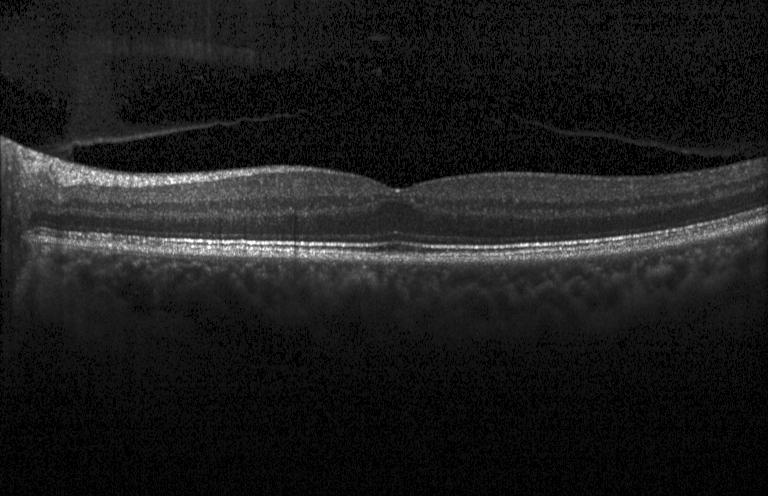 Optical coherence tomography scan. Impression: no evidence of choroidal neovascularization, diabetic macular edema, or drusen.